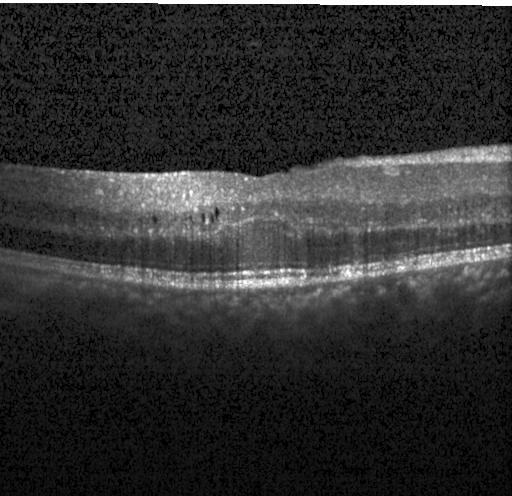

OCT line scan. Finding: diabetic macular edema.